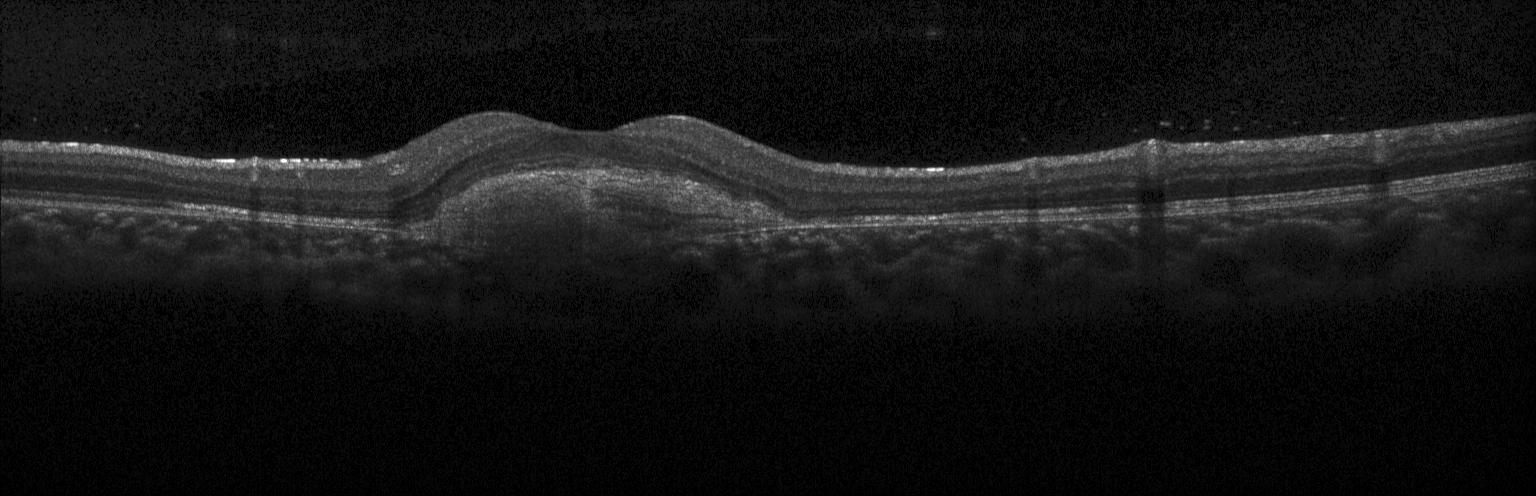
Heidelberg Spectralis. Optical coherence tomography scan.
Impression: choroidal neovascularization (CNV).